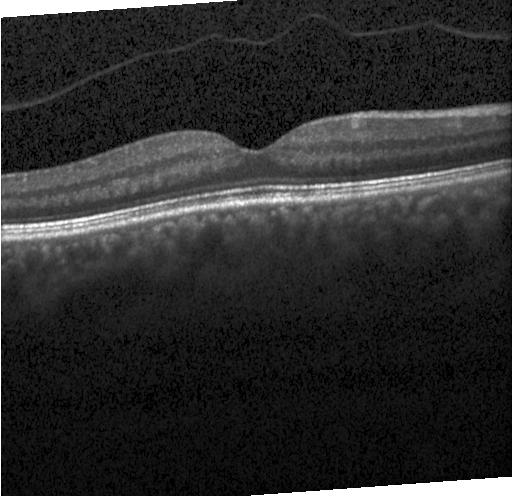 Dx: no choroidal neovascularization, no diabetic macular edema, and no drusen.